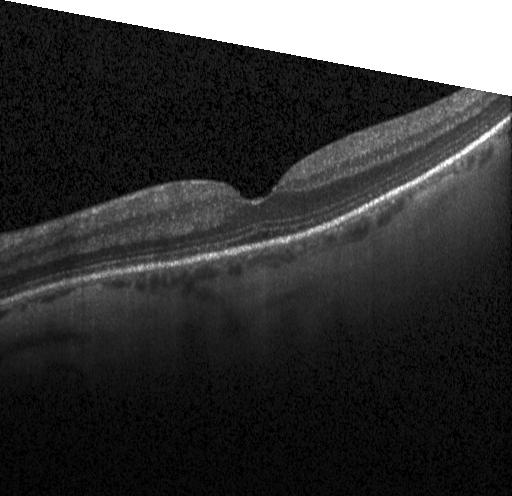

Through the macula. OCT line scan. Spectral-domain optical coherence tomography. Acquired on a Heidelberg Spectralis.
Diagnosis: no choroidal neovascularization, no diabetic macular edema, and no drusen.